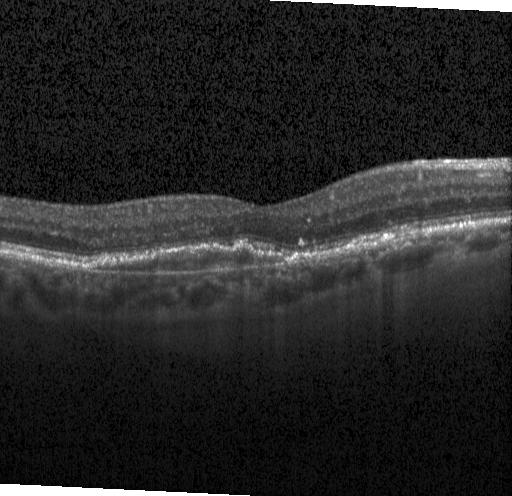
Centered on the fovea; spectral-domain optical coherence tomography; optical coherence tomography B-scan; Heidelberg Spectralis.
Macular OCT: choroidal neovascularization.